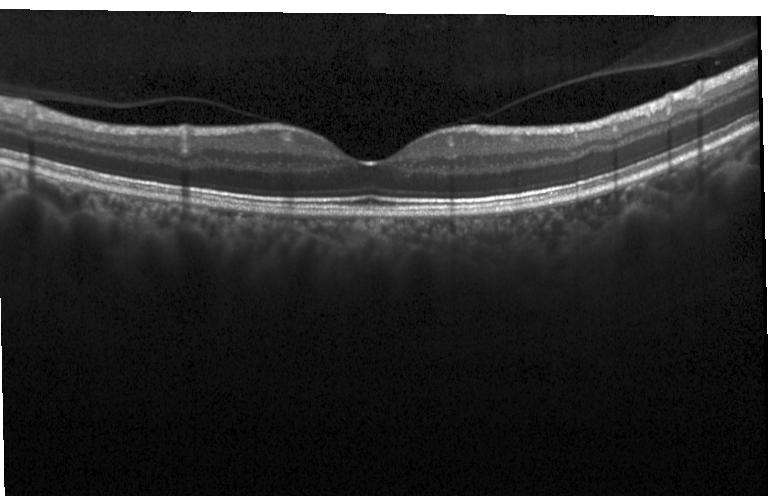
OCT line scan.
Impression: no CNV, no DME, and no drusen.